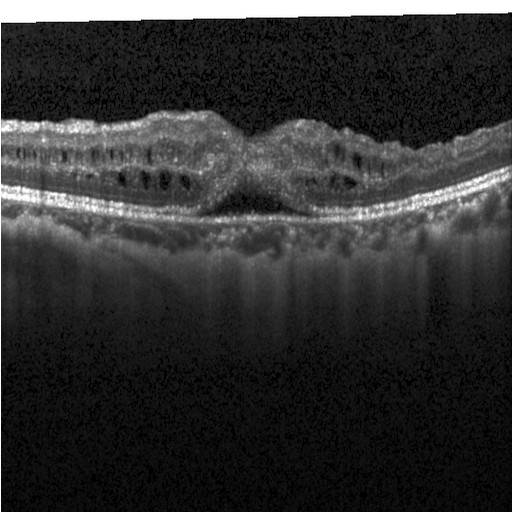

Finding: diabetic macular edema.